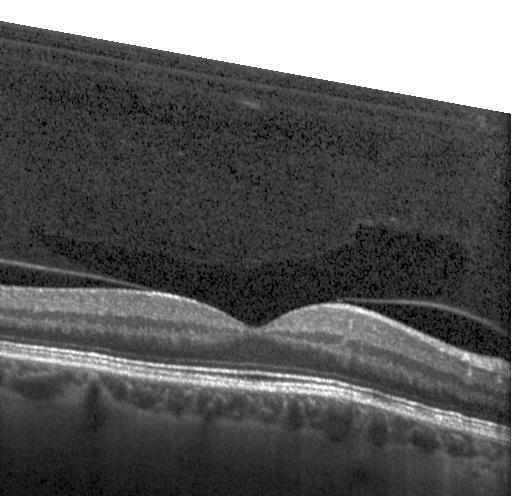

Acquired on a Heidelberg Spectralis · OCT B-scan · SD-OCT · macular scan — Finding: no CNV, no DME, and no drusen.